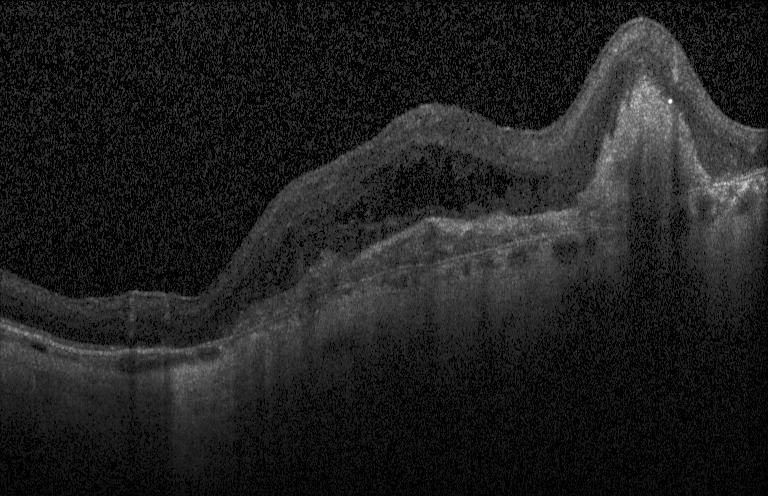
Finding: CNV.